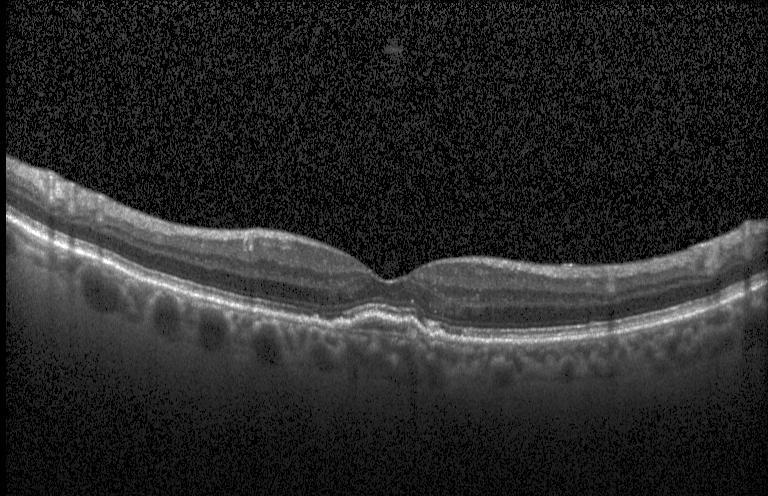

Instrument: Heidelberg Spectralis. Through the macula. Retinal OCT B-scan. Spectral-domain optical coherence tomography
Dx: a choroidal neovascular membrane.